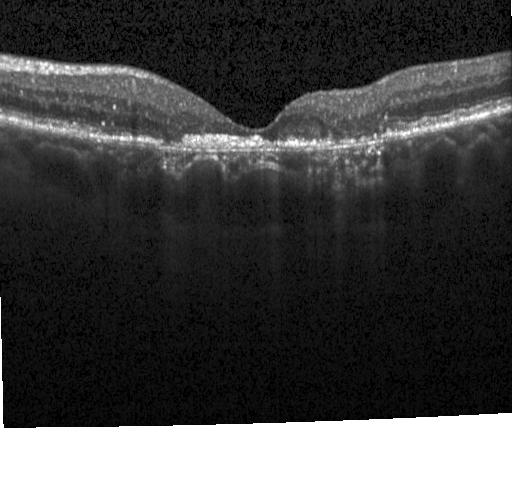

Spectral-domain OCT · horizontal scan through the fovea · Heidelberg Spectralis OCT system · optical coherence tomography B-scan
Diagnosis: choroidal neovascularization (CNV).